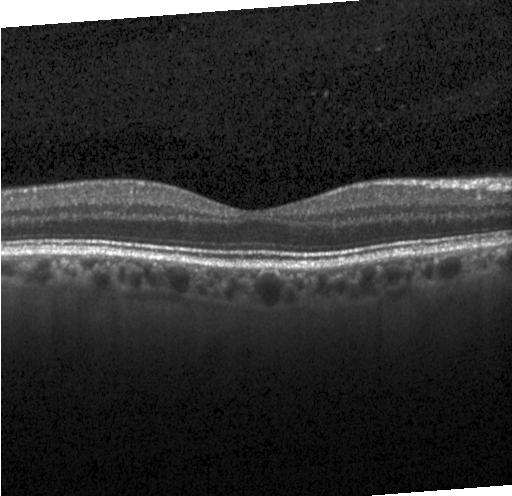
Heidelberg Spectralis. OCT B-scan
Dx: no CNV, DME, or drusen.